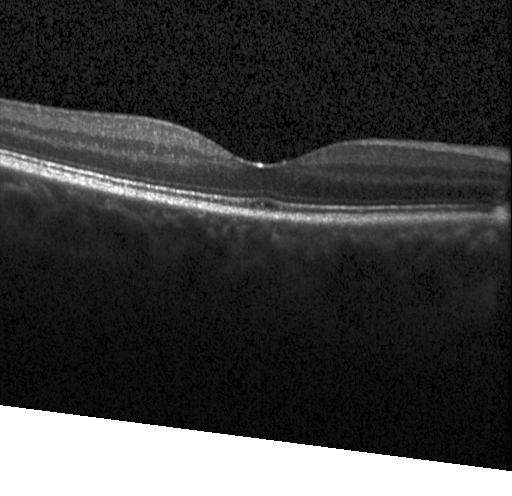
Centered on the fovea · Heidelberg Spectralis · spectral-domain OCT · retinal OCT cross-section
Assessment: neither CNV, DME, nor drusen.